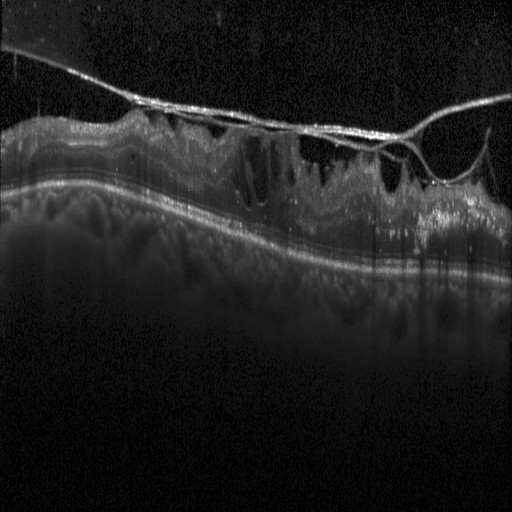 OCT finding: diabetic macular edema.